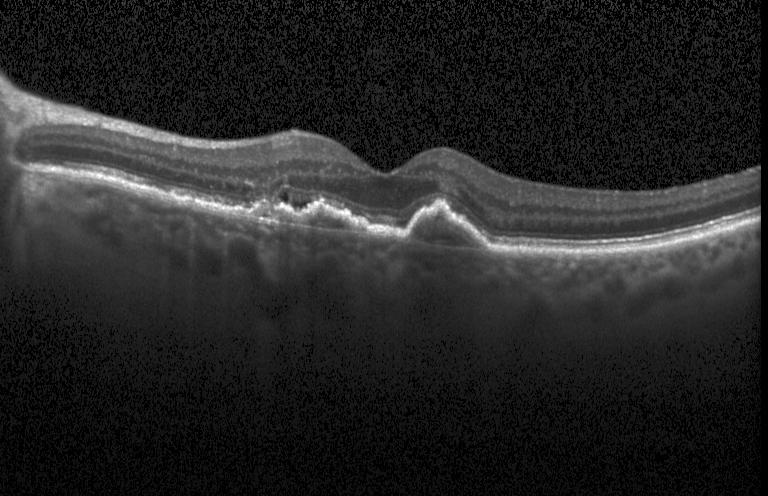

Centered on the fovea · instrument: Heidelberg Spectralis · optical coherence tomography scan.
Finding: a choroidal neovascular membrane.